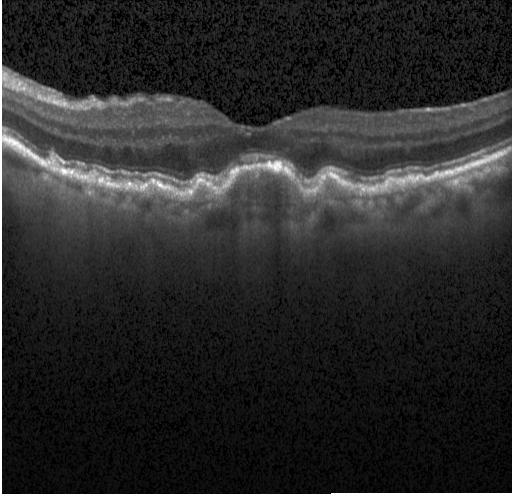

Diagnosis: a choroidal neovascular membrane.